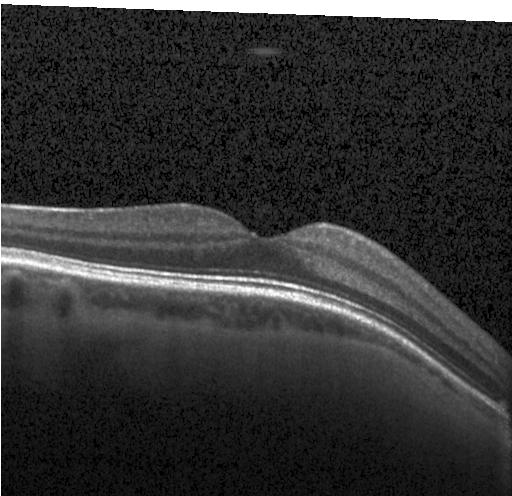
Retinal OCT B-scan.
This B-scan demonstrates no evidence of choroidal neovascularization, diabetic macular edema, or drusen.